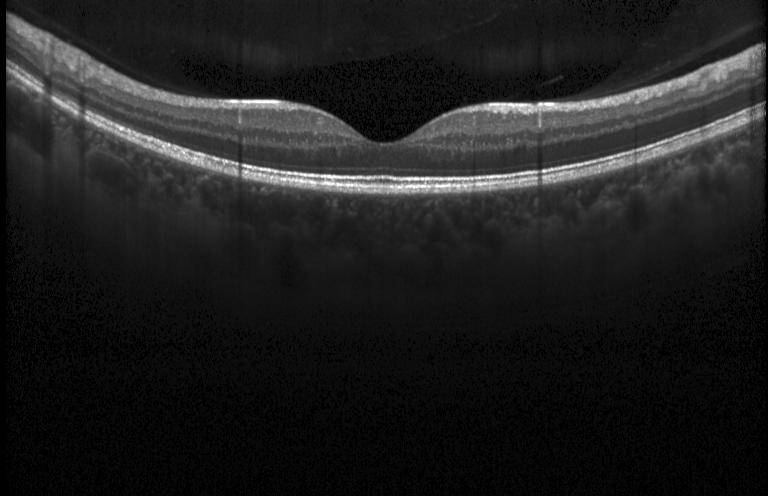 Impression: no CNV, no DME, and no drusen.